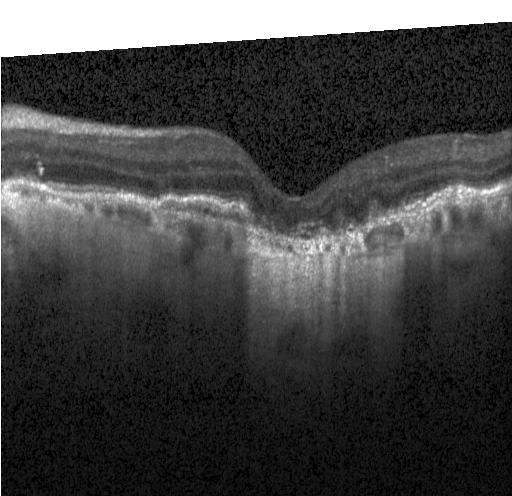 Retinal OCT cross-section, spectral-domain OCT — Macular OCT: choroidal neovascularization (CNV).